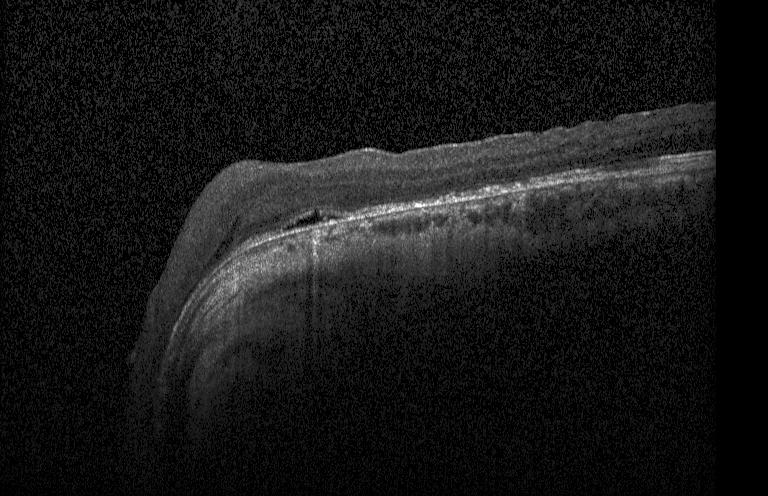
Spectral-domain optical coherence tomography · optical coherence tomography scan · instrument: Heidelberg Spectralis. OCT finding: choroidal neovascularization.